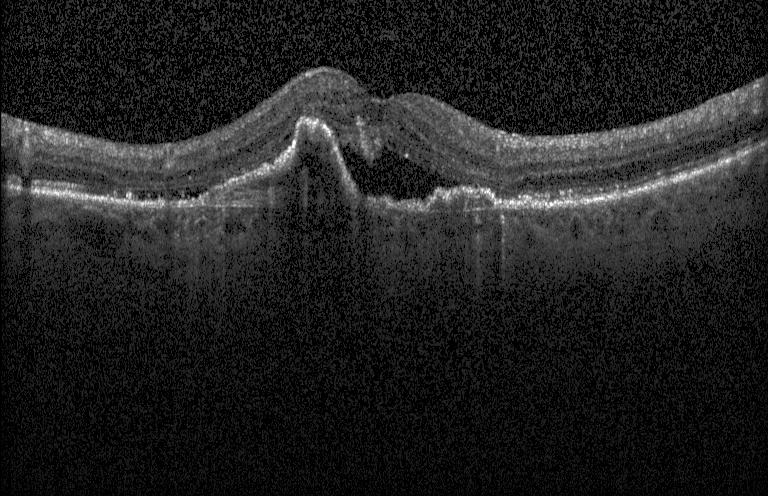

Centered on the fovea; OCT line scan; instrument: Heidelberg Spectralis; spectral-domain OCT
Diagnosis: CNV.